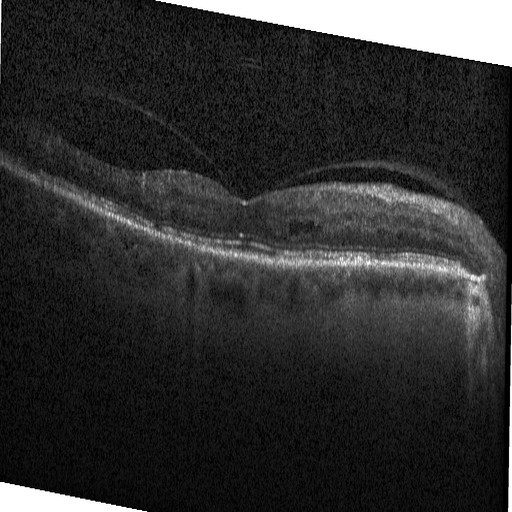

Fovea-centered · spectral-domain optical coherence tomography · optical coherence tomography scan · acquired on a Heidelberg Spectralis. Diagnosis: diabetic macular edema.